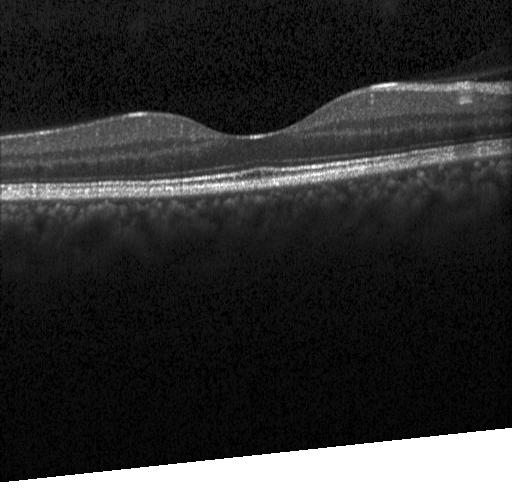 Horizontal scan through the fovea, retinal OCT cross-section.
Macular OCT: no CNV, DME, or drusen.